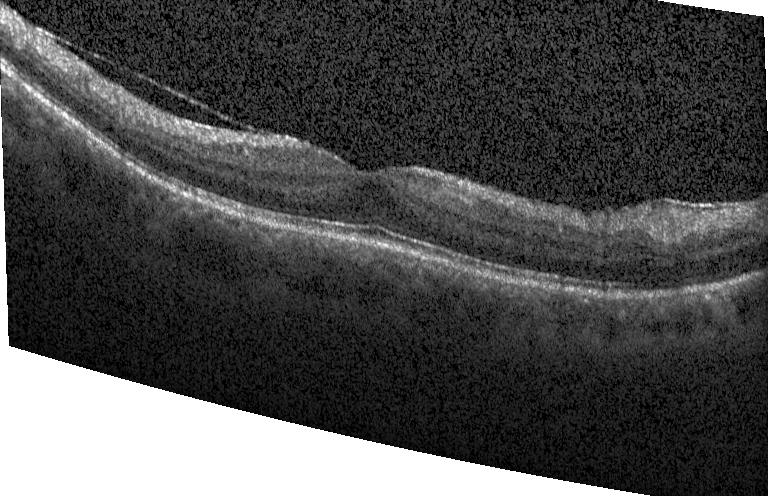 Diagnosis: neither choroidal neovascularization, diabetic macular edema, nor drusen.